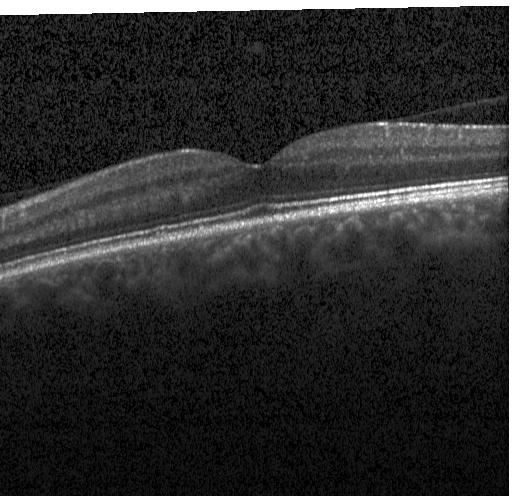
Retinal OCT cross-section. Macular scan.
Impression: neither CNV, DME, nor drusen.